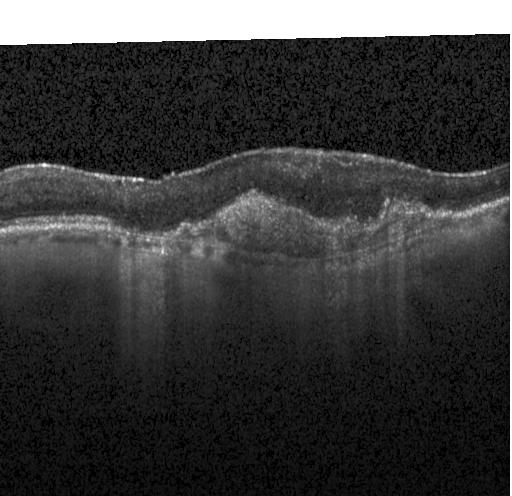 Spectral-domain optical coherence tomography. OCT B-scan — Finding: a choroidal neovascular membrane.